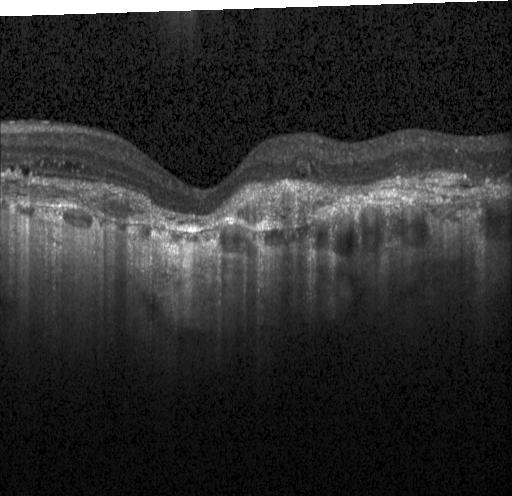

This B-scan demonstrates a choroidal neovascular membrane.